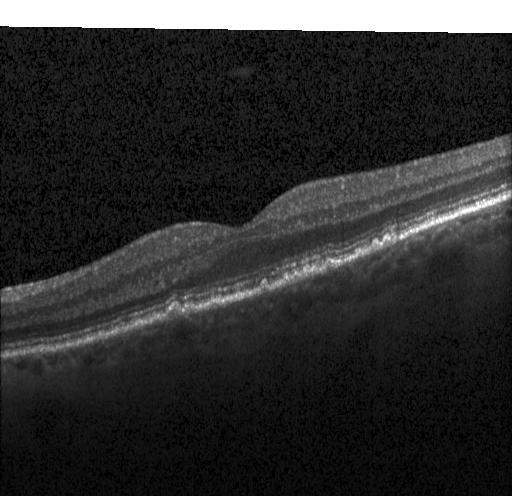
Fovea-centered · optical coherence tomography B-scan — Finding: multiple drusen.